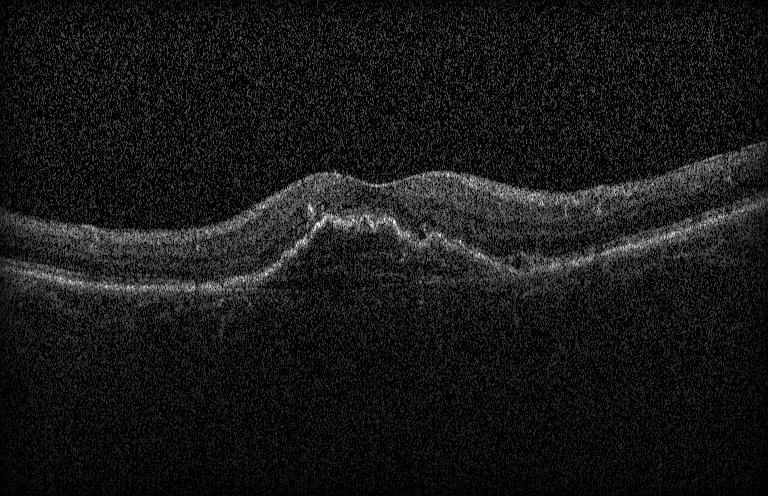

Spectral-domain OCT, retinal OCT B-scan
Assessment: choroidal neovascularization (CNV).